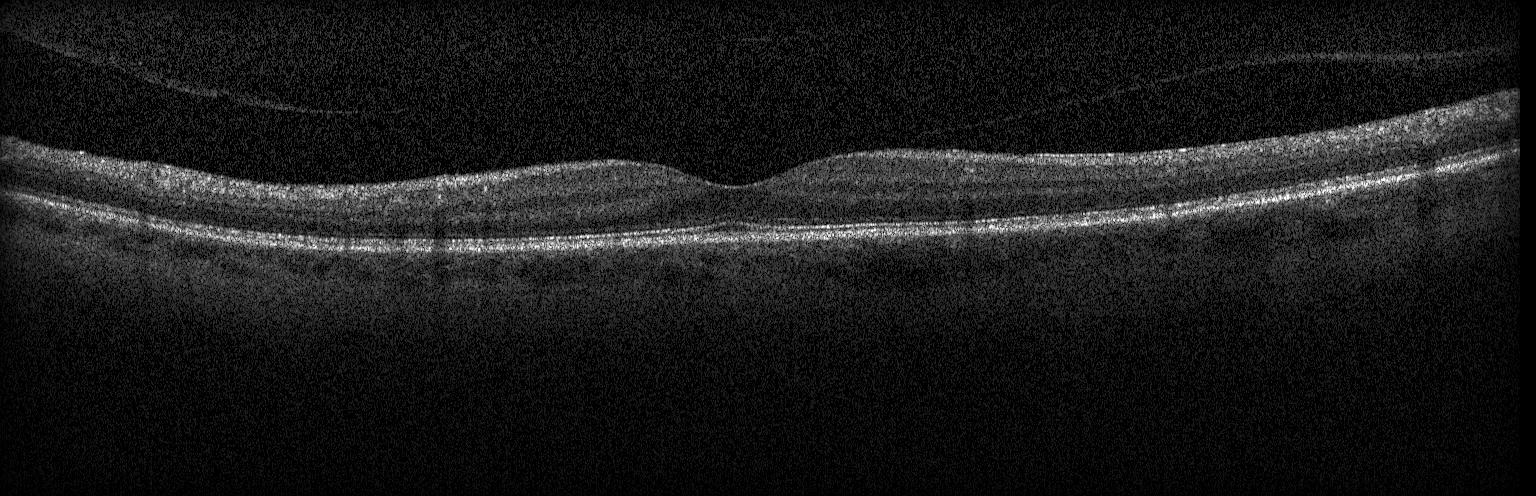

Optical coherence tomography B-scan · through the macula · instrument: Heidelberg Spectralis · spectral-domain optical coherence tomography. Macular OCT: neither choroidal neovascularization, diabetic macular edema, nor drusen.